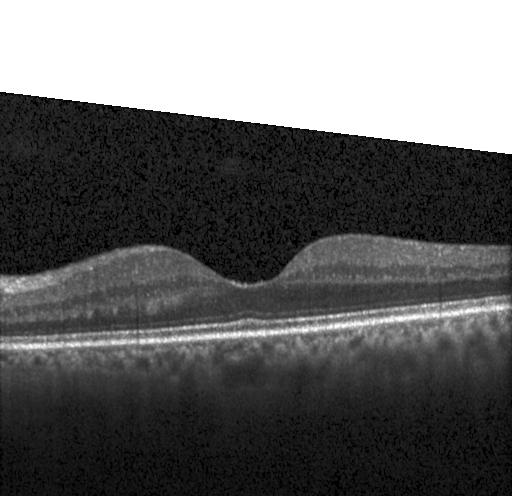 OCT line scan — Impression: neither choroidal neovascularization, diabetic macular edema, nor drusen.